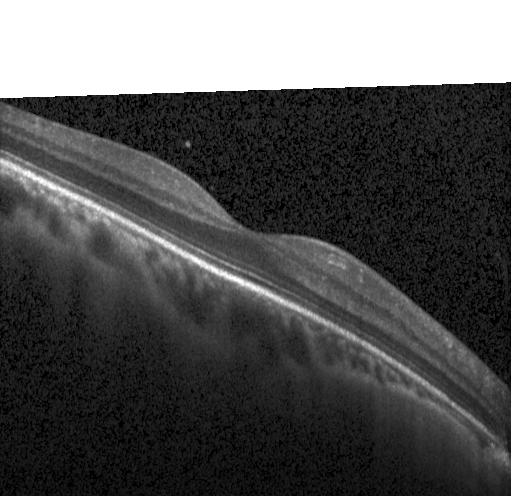

Retinal OCT B-scan; SD-OCT; macular scan — This B-scan demonstrates no evidence of CNV, DME, or drusen.